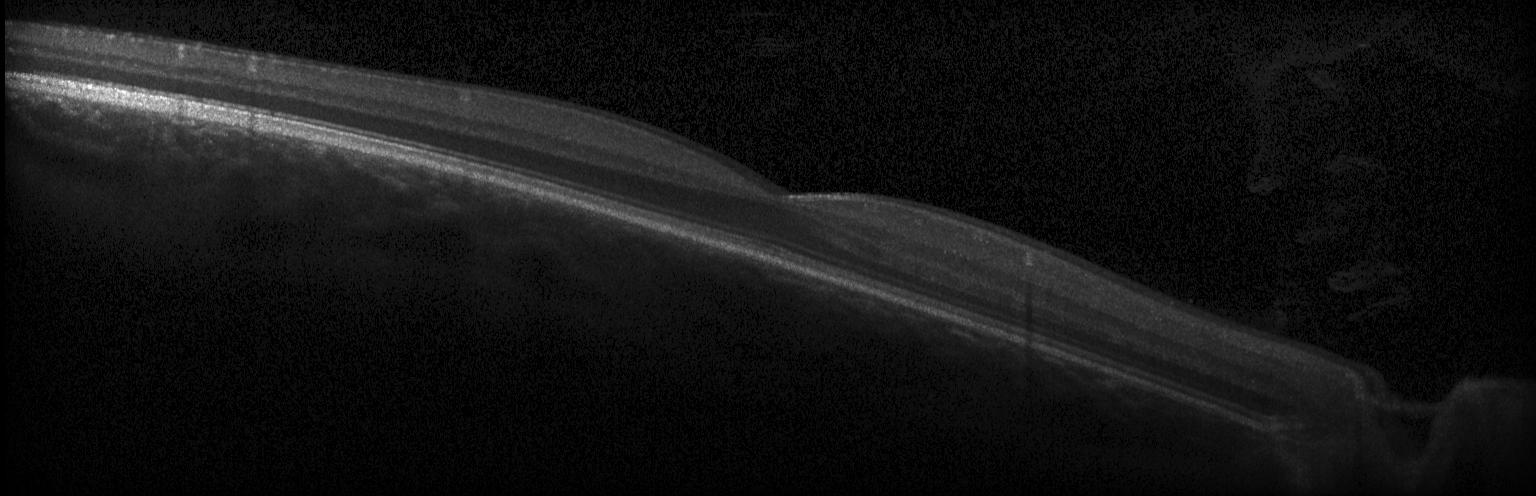

No CNV, no DME, and no drusen.